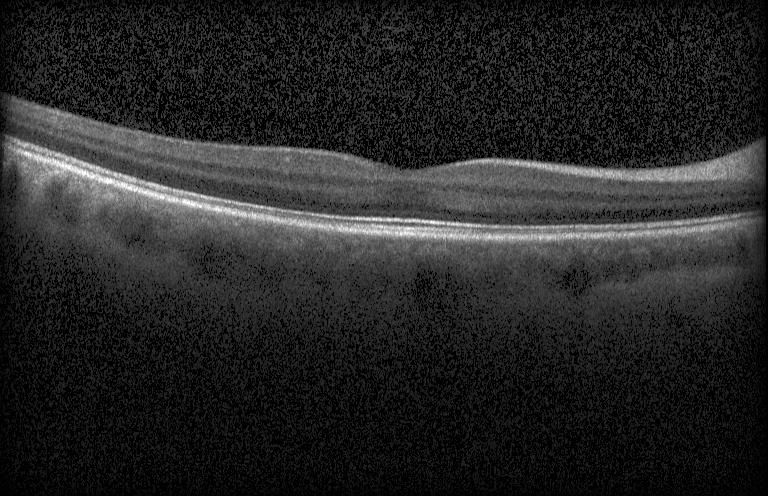

Acquired on a Heidelberg Spectralis · SD-OCT · optical coherence tomography B-scan · fovea-centered
Finding: no evidence of choroidal neovascularization, diabetic macular edema, or drusen.